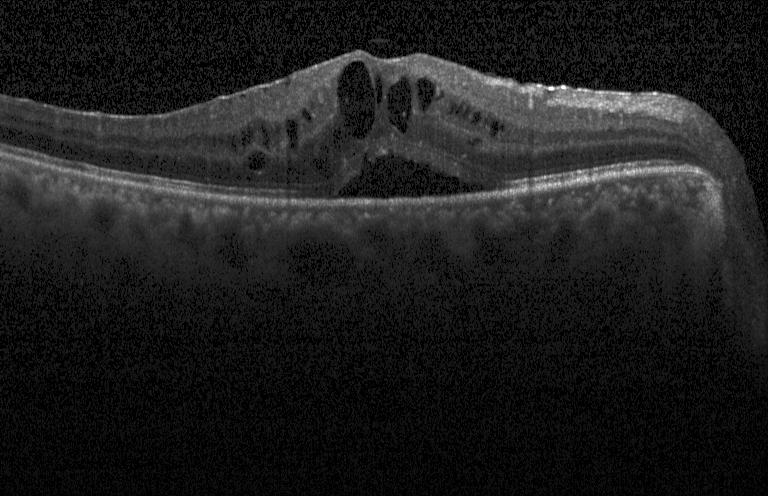

Diagnosis: DME.